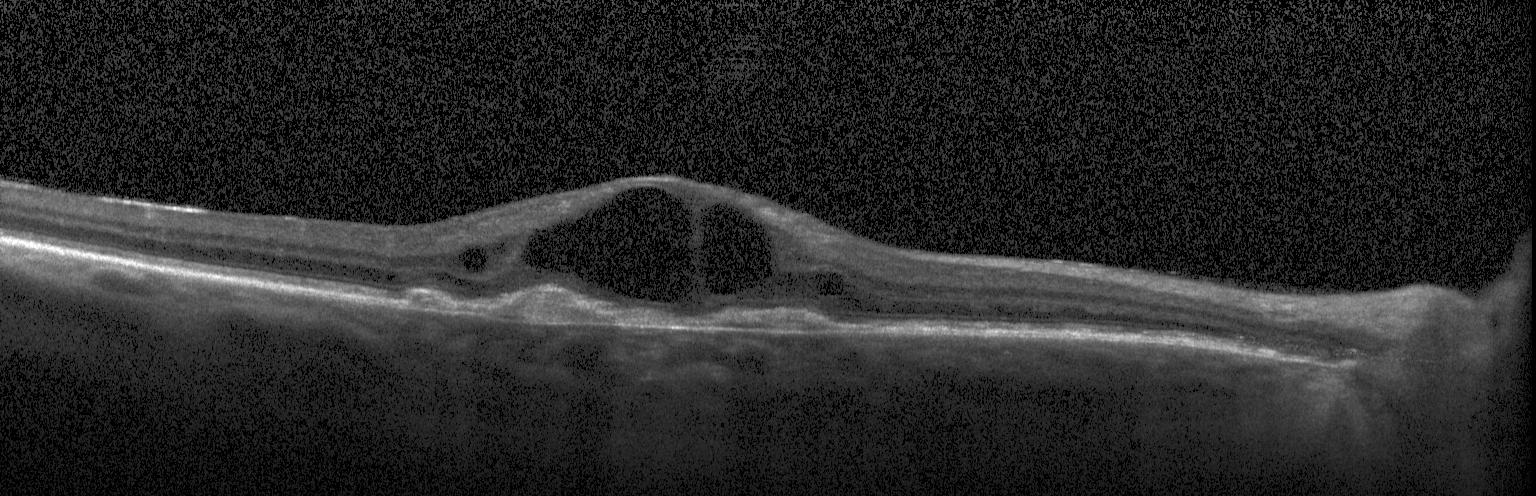
Optical coherence tomography B-scan. Macular OCT: choroidal neovascularization.